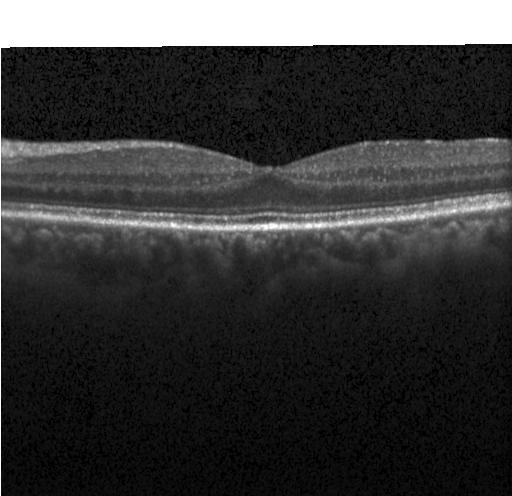

SD-OCT. Through the macula. OCT line scan. Heidelberg Spectralis.
Diagnosis: no choroidal neovascularization, diabetic macular edema, or drusen.